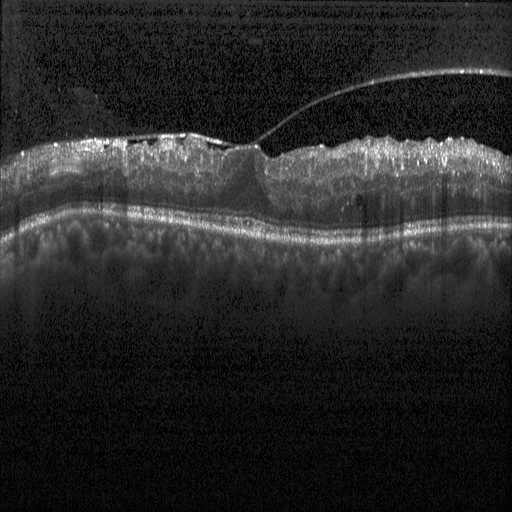

OCT finding: diabetic macular edema (DME).